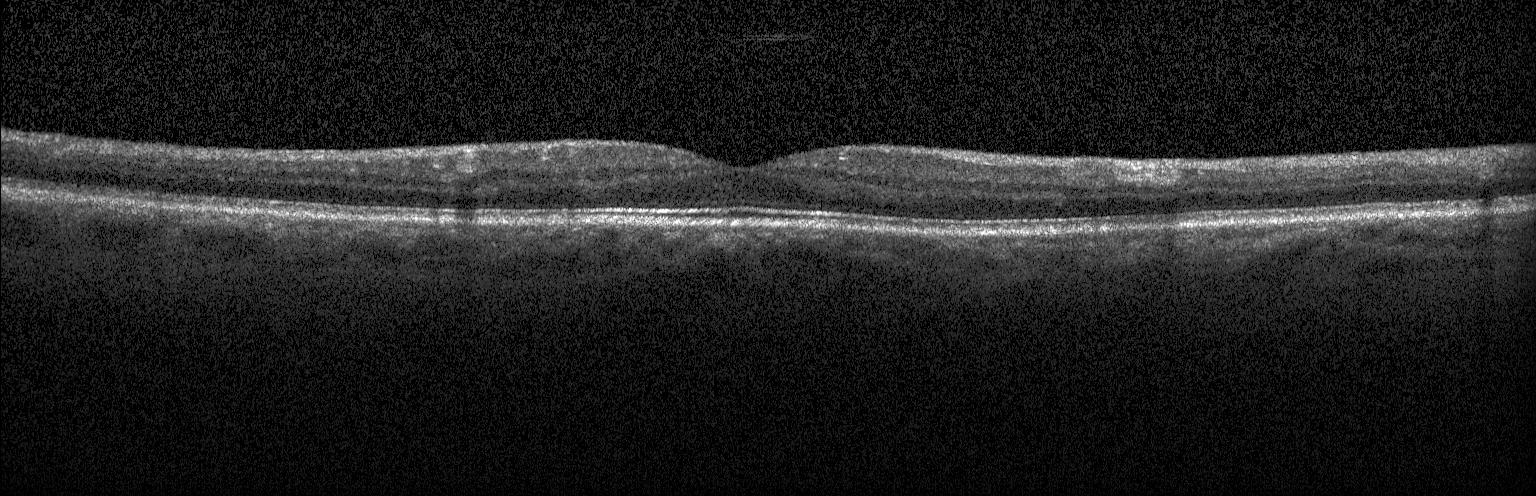
Spectral-domain OCT; Heidelberg Spectralis; optical coherence tomography scan. The scan shows no evidence of choroidal neovascularization, diabetic macular edema, or drusen.